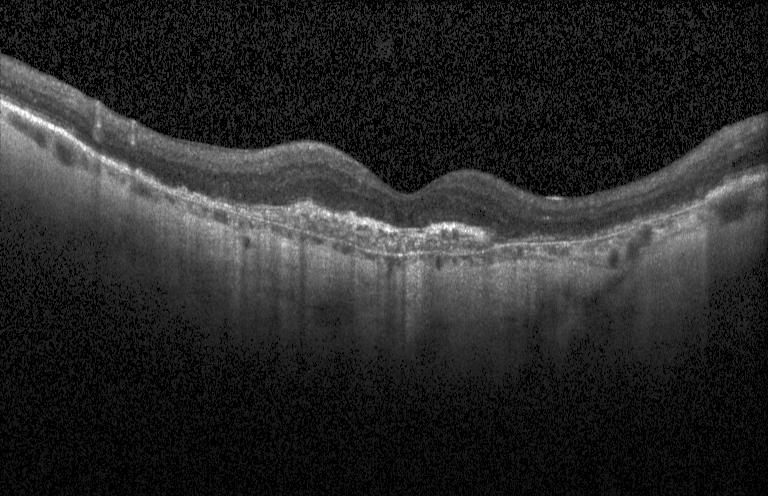
Heidelberg Spectralis OCT system; SD-OCT; retinal OCT cross-section; through the macula
Finding: a choroidal neovascular membrane.